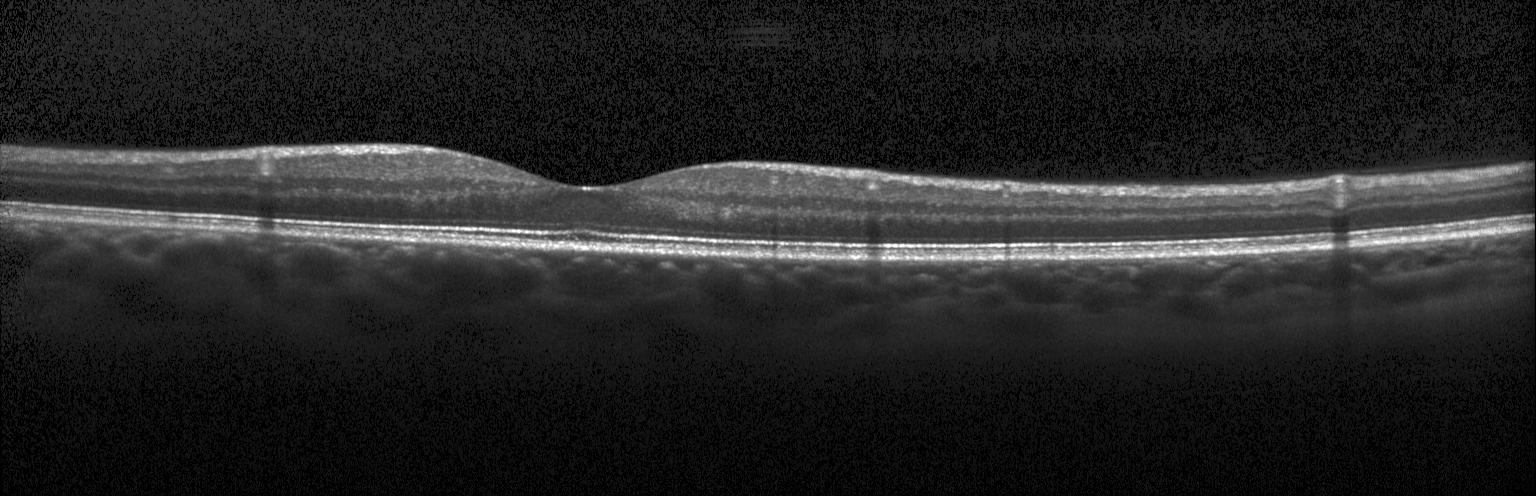
Macular scan. SD-OCT. OCT line scan — Diagnosis: no choroidal neovascularization, no diabetic macular edema, and no drusen.